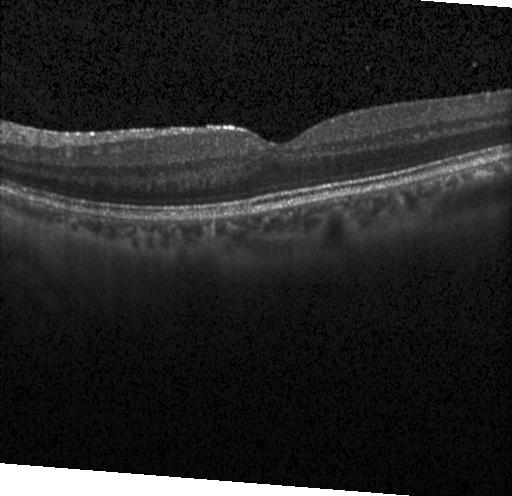 Macular OCT: no evidence of choroidal neovascularization, diabetic macular edema, or drusen.